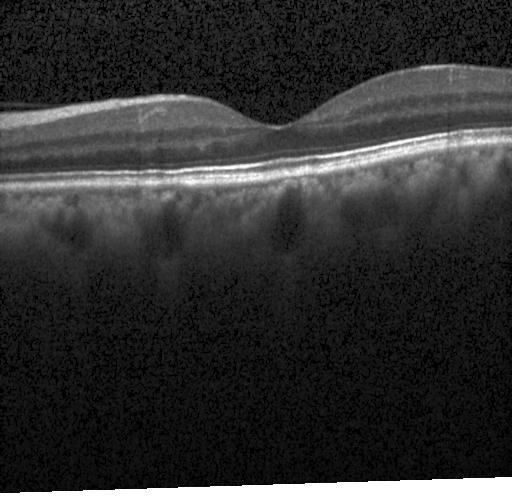

Dx: no choroidal neovascularization, diabetic macular edema, or drusen.